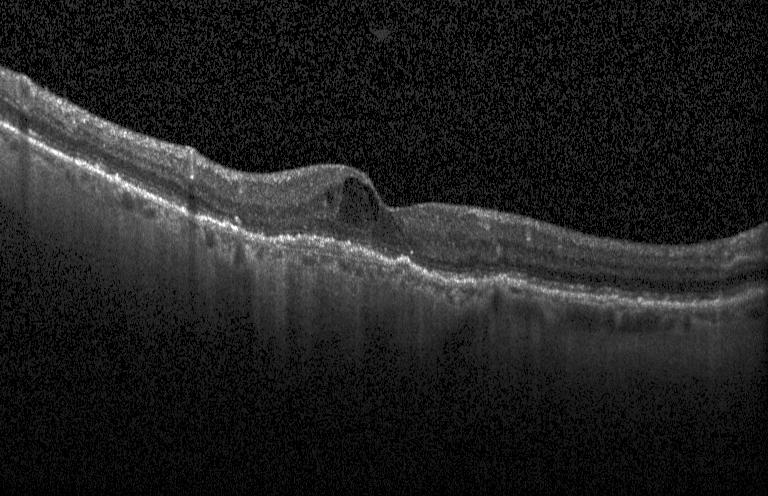 Retinal OCT cross-section · spectral-domain optical coherence tomography · through the macula
Diagnosis: a choroidal neovascular membrane.